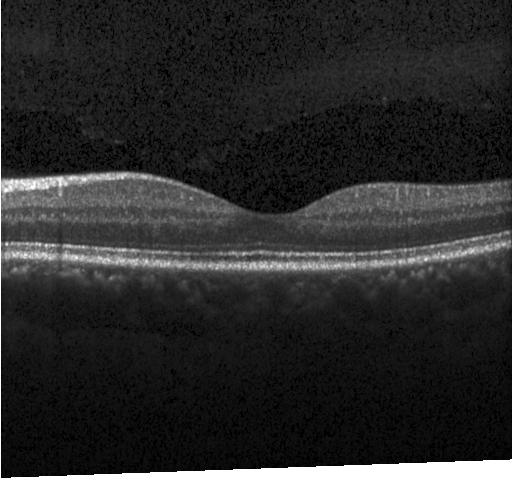
Impression: no evidence of choroidal neovascularization, diabetic macular edema, or drusen.